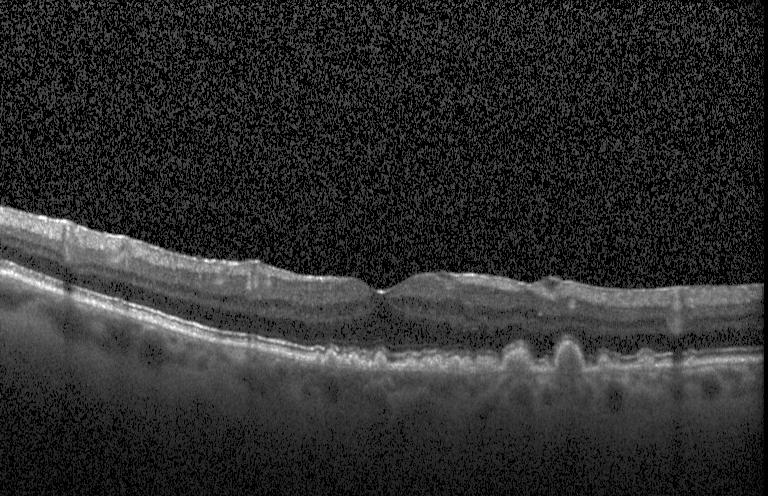

Horizontal scan through the fovea. OCT line scan. Spectral-domain OCT. Heidelberg Spectralis OCT system — Assessment: multiple drusen.